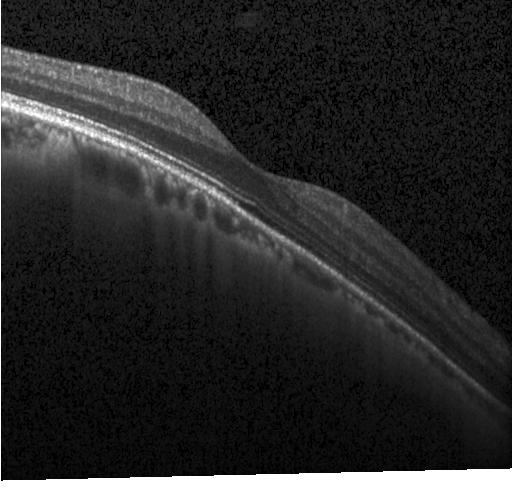
Optical coherence tomography B-scan; SD-OCT; instrument: Heidelberg Spectralis; horizontal scan through the fovea — No CNV, DME, or drusen.